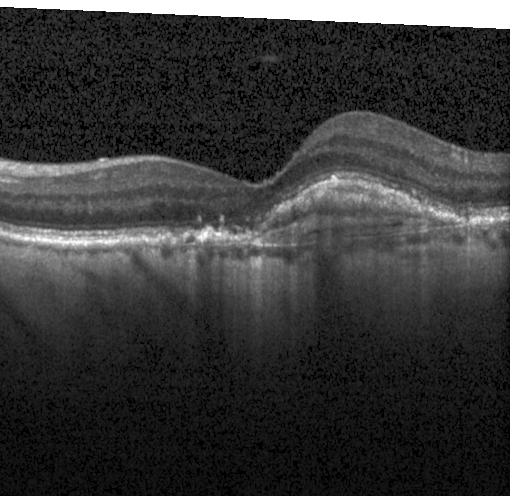
Instrument: Heidelberg Spectralis, centered on the fovea, retinal OCT B-scan.
Impression: choroidal neovascularization.